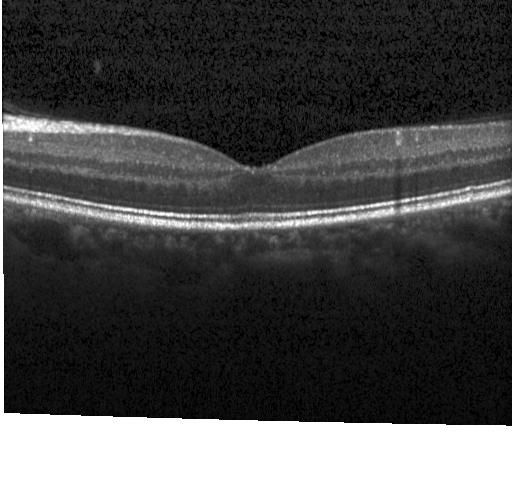
SD-OCT; centered on the fovea; instrument: Heidelberg Spectralis; retinal OCT B-scan
Diagnosis: no choroidal neovascularization, diabetic macular edema, or drusen.